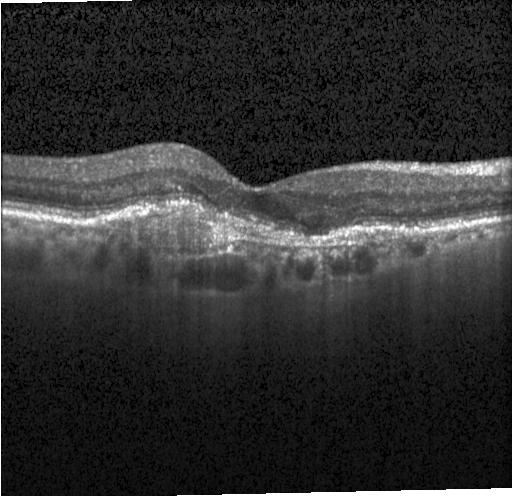
Spectral-domain optical coherence tomography, macular scan, OCT B-scan. OCT finding: a choroidal neovascular membrane.